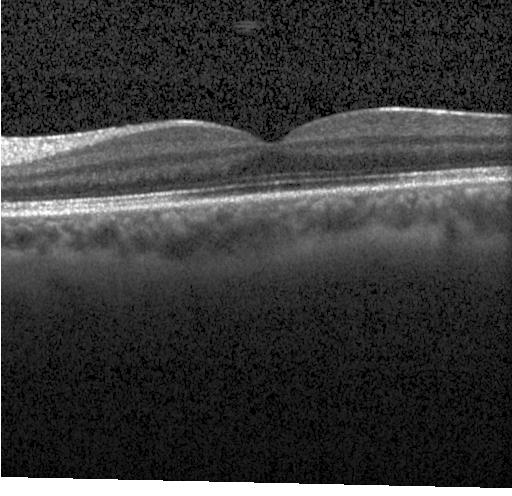

Retinal OCT cross-section · through the macula · spectral-domain OCT · Heidelberg Spectralis. Macular OCT: neither CNV, DME, nor drusen.